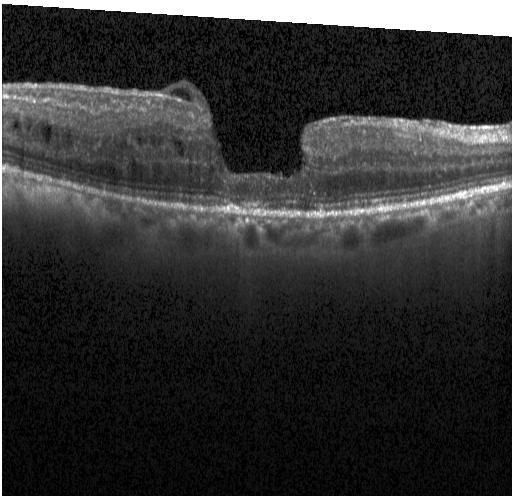
OCT B-scan showing diabetic macular edema (DME).